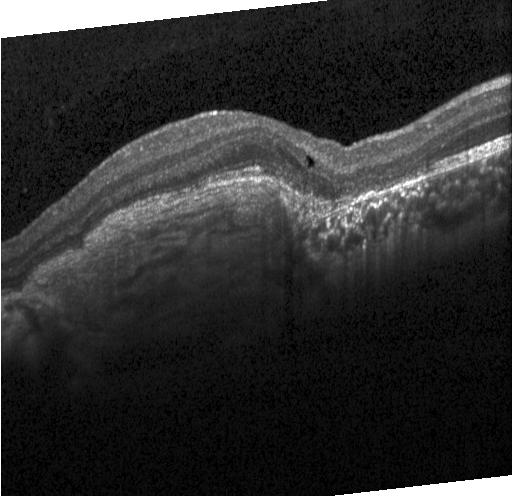

Heidelberg Spectralis; fovea-centered; optical coherence tomography scan — OCT finding: choroidal neovascularization.